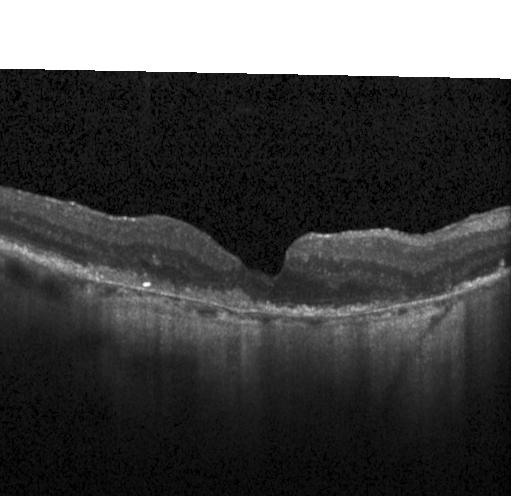

OCT line scan. The scan shows a choroidal neovascular membrane.